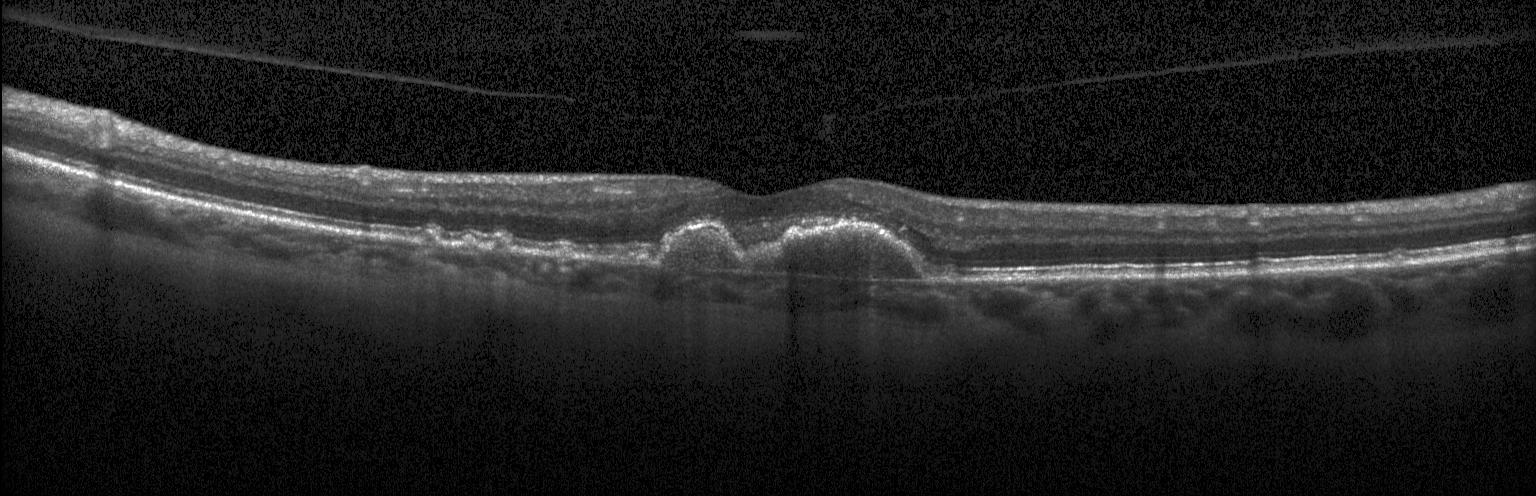
Diagnosis: choroidal neovascularization (CNV).